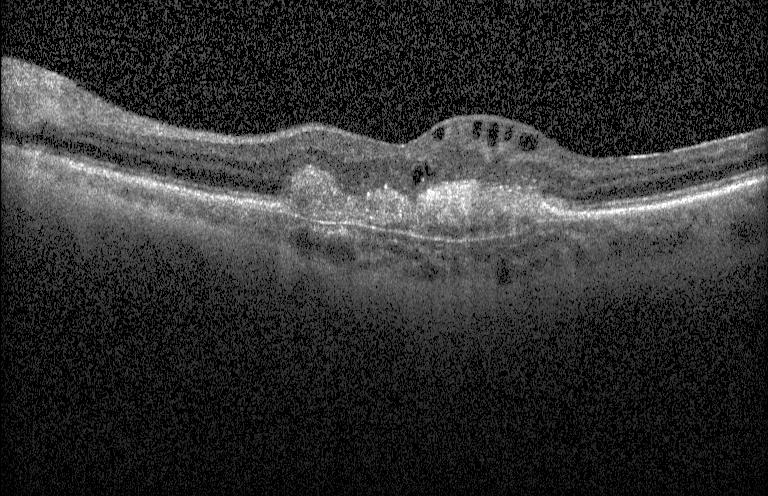 Spectral-domain OCT · optical coherence tomography scan · Heidelberg Spectralis · centered on the fovea.
Impression: choroidal neovascularization (CNV).